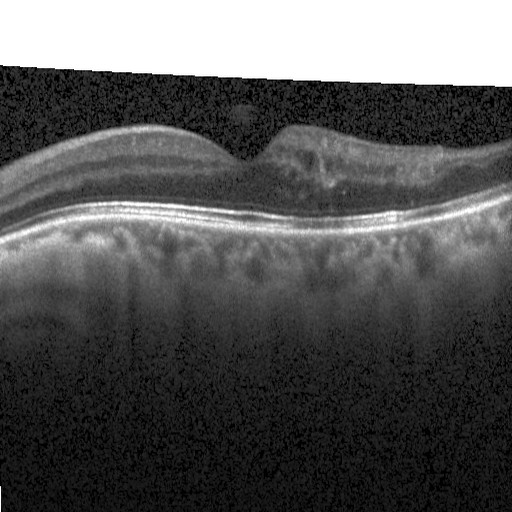 Fovea-centered; retinal OCT B-scan; SD-OCT.
Finding: DME.